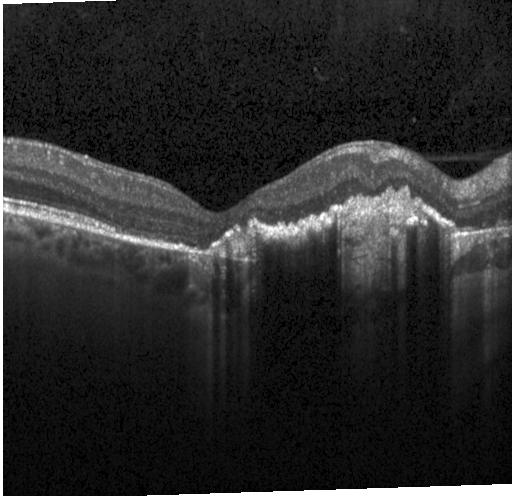

This B-scan demonstrates choroidal neovascularization (CNV).